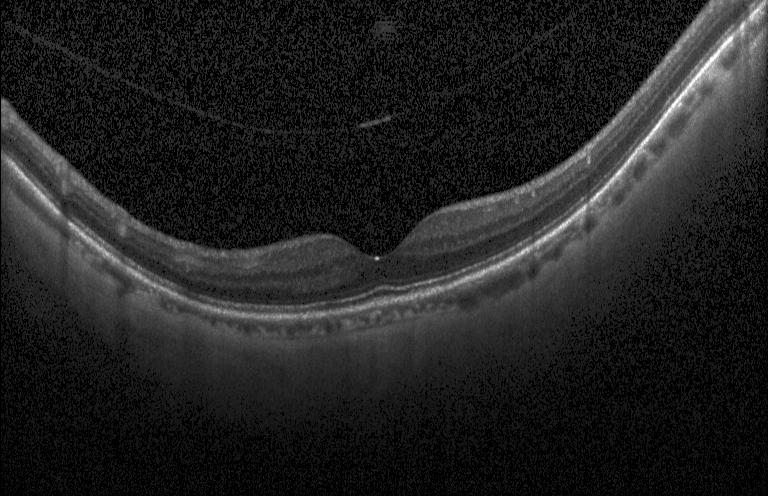
OCT line scan — Dx: no choroidal neovascularization, diabetic macular edema, or drusen.